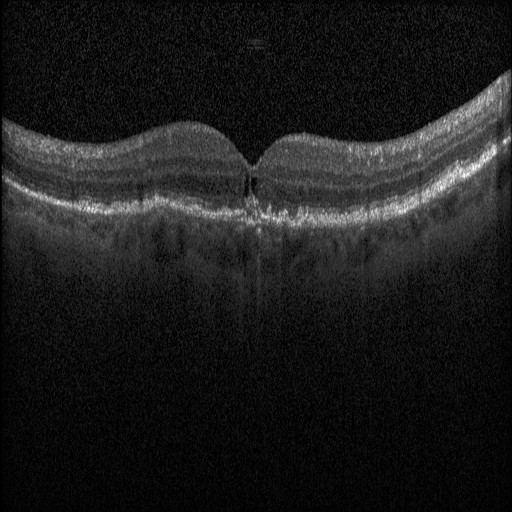 OCT line scan. Horizontal scan through the fovea. Acquired on a Heidelberg Spectralis.
Diabetic macular edema (DME).